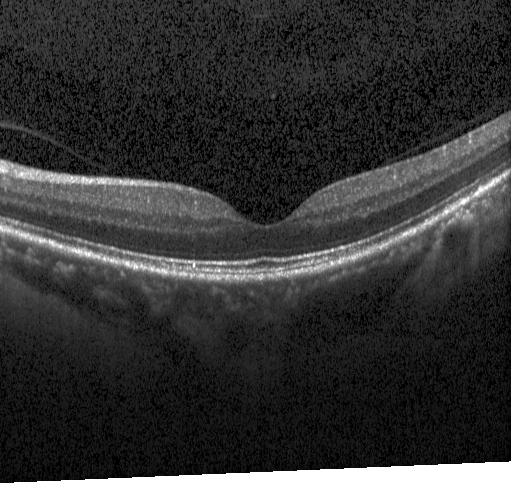

Optical coherence tomography scan, horizontal scan through the fovea, Heidelberg Spectralis OCT system
No evidence of choroidal neovascularization, diabetic macular edema, or drusen.